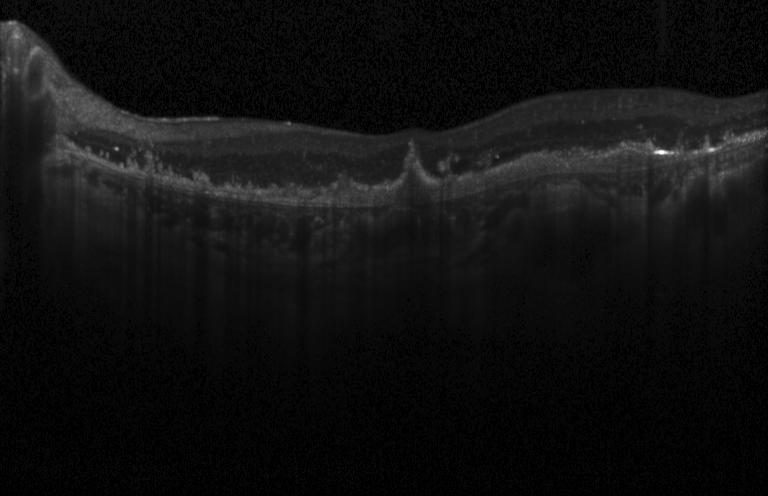 OCT finding: choroidal neovascularization.